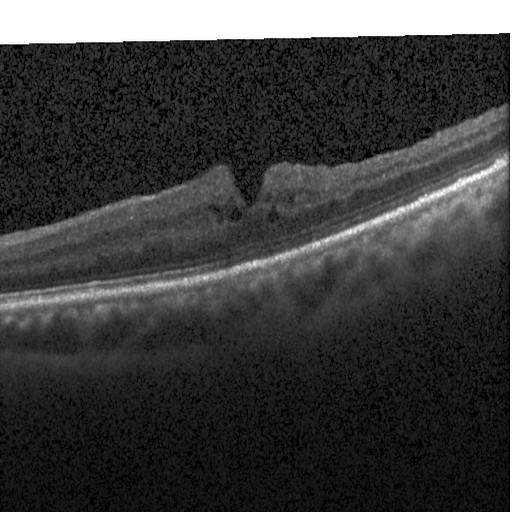 Retinal OCT cross-section. Finding: diabetic macular edema.